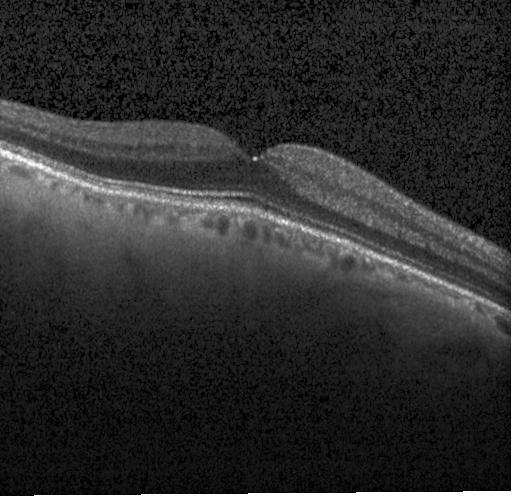 Retinal OCT cross-section — Assessment: no evidence of CNV, DME, or drusen.